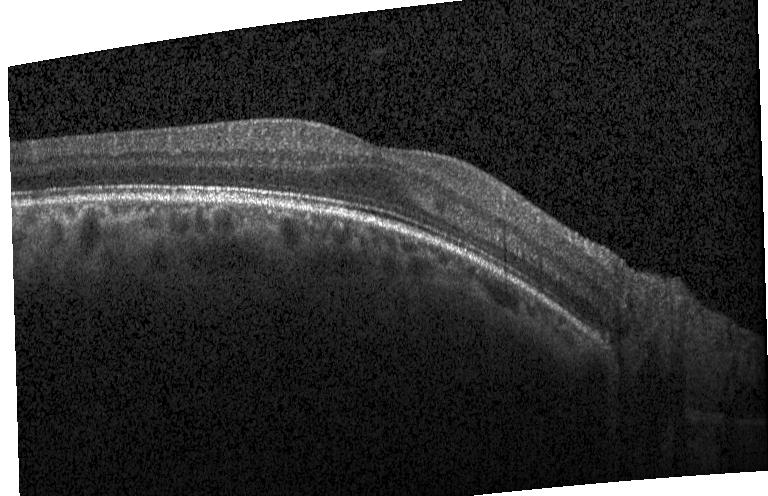
Centered on the fovea; OCT line scan; spectral-domain optical coherence tomography; Heidelberg Spectralis OCT system.
Macular OCT: no evidence of choroidal neovascularization, diabetic macular edema, or drusen.